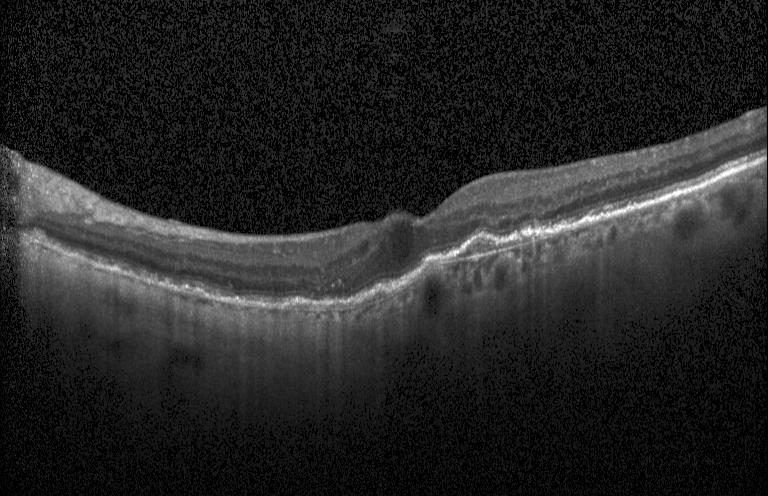

OCT line scan.
Macular OCT: a choroidal neovascular membrane.